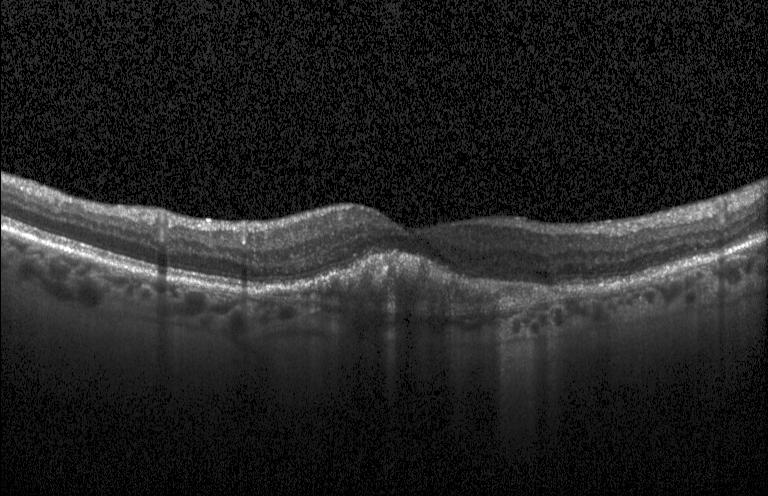

Spectral-domain OCT; through the macula; optical coherence tomography B-scan
The scan shows choroidal neovascularization.